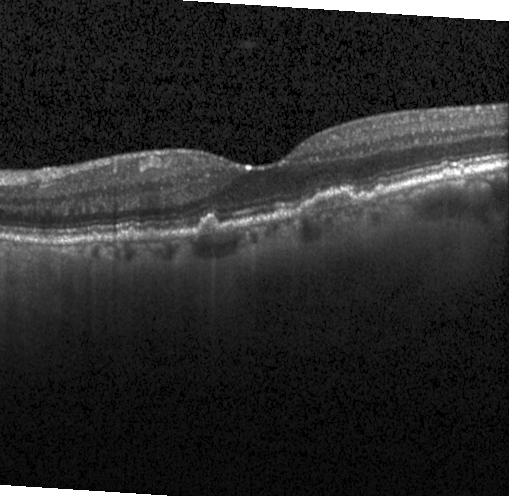 Heidelberg Spectralis, retinal OCT B-scan, spectral-domain OCT
Finding: multiple drusen.